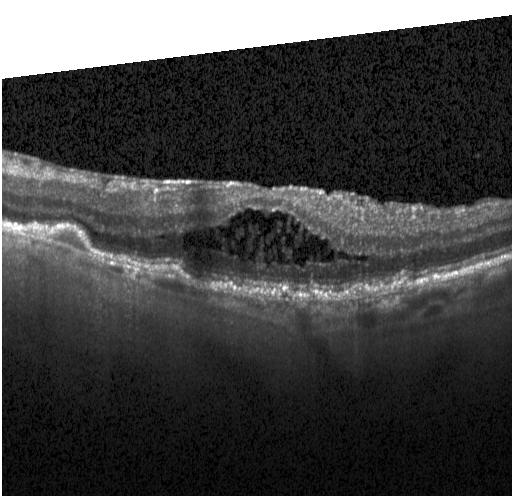

This B-scan demonstrates DME.